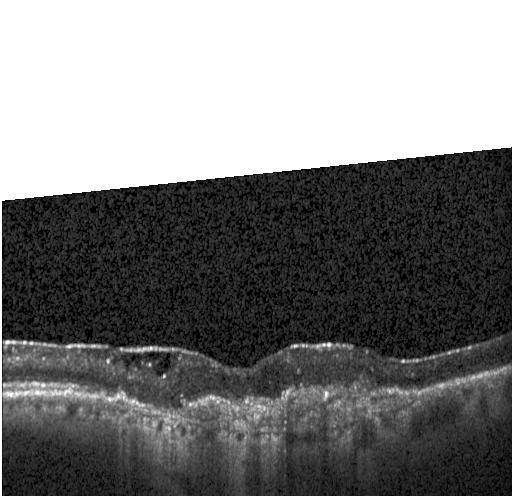

Spectral-domain OCT, optical coherence tomography scan, Heidelberg Spectralis OCT system, centered on the fovea
Assessment: CNV.